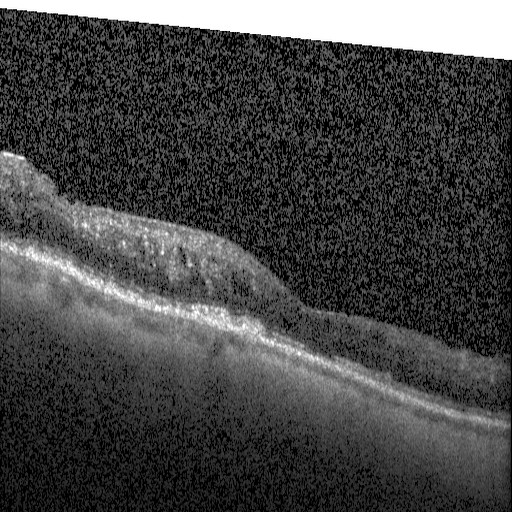
Instrument: Heidelberg Spectralis · fovea-centered · spectral-domain optical coherence tomography · optical coherence tomography scan.
Impression: DME.